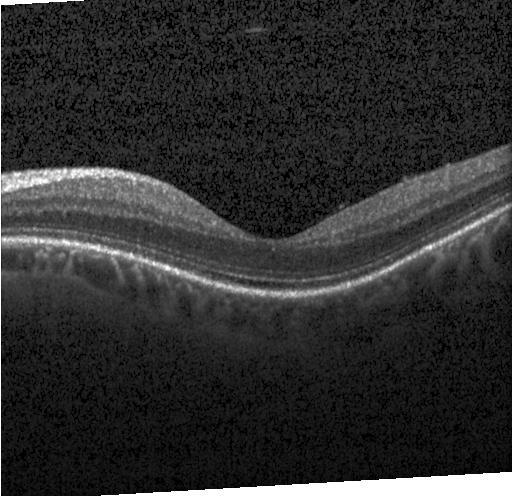 Heidelberg Spectralis OCT system; centered on the fovea; SD-OCT; retinal OCT B-scan
This B-scan demonstrates no evidence of choroidal neovascularization, diabetic macular edema, or drusen.